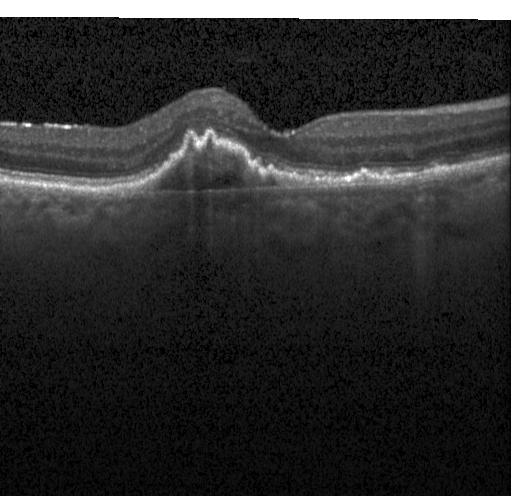

Spectral-domain OCT; retinal OCT B-scan.
OCT finding: choroidal neovascularization.